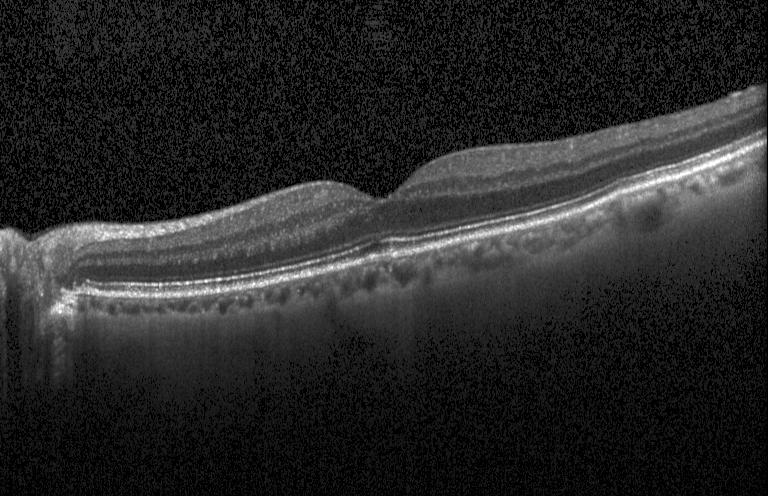
Retinal OCT cross-section · acquired on a Heidelberg Spectralis. Assessment: no evidence of CNV, DME, or drusen.